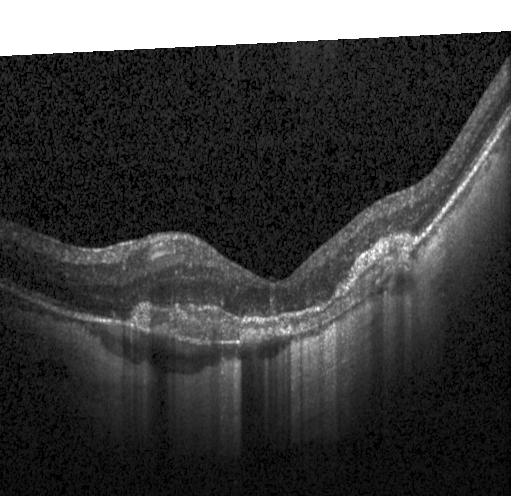

Assessment: a choroidal neovascular membrane.